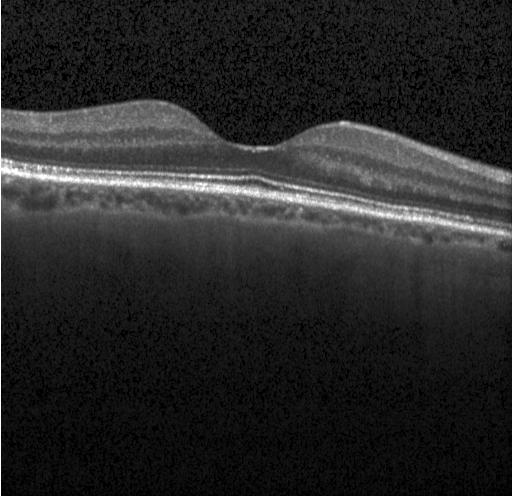

No CNV, no DME, and no drusen.